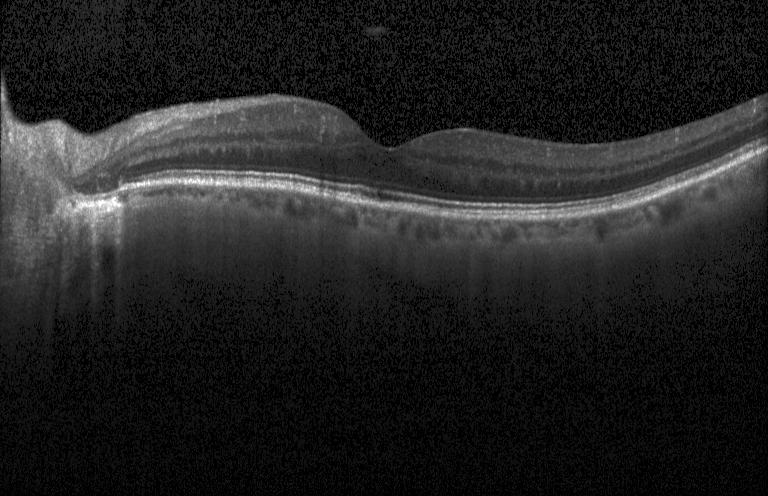 Optical coherence tomography B-scan · SD-OCT · instrument: Heidelberg Spectralis — Diagnosis: no choroidal neovascularization, diabetic macular edema, or drusen.